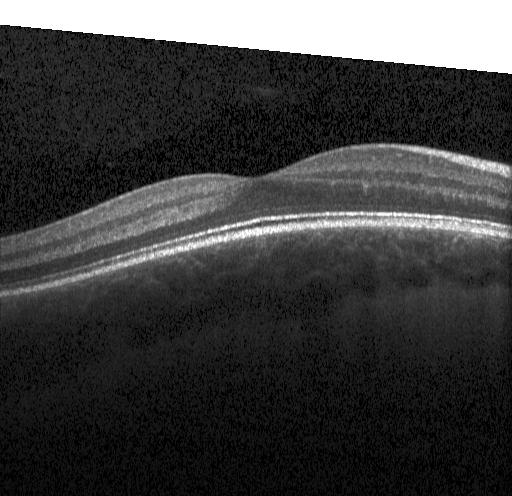
Finding: no choroidal neovascularization, no diabetic macular edema, and no drusen.